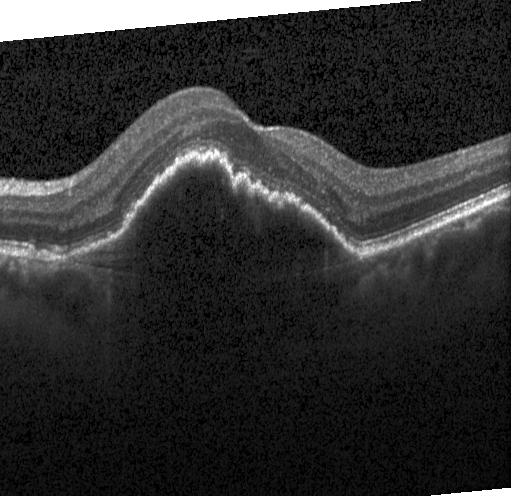
Diagnosis: a choroidal neovascular membrane.